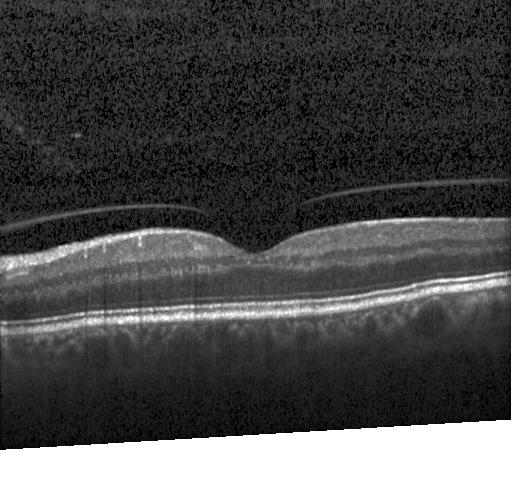 Diagnosis: neither choroidal neovascularization, diabetic macular edema, nor drusen.